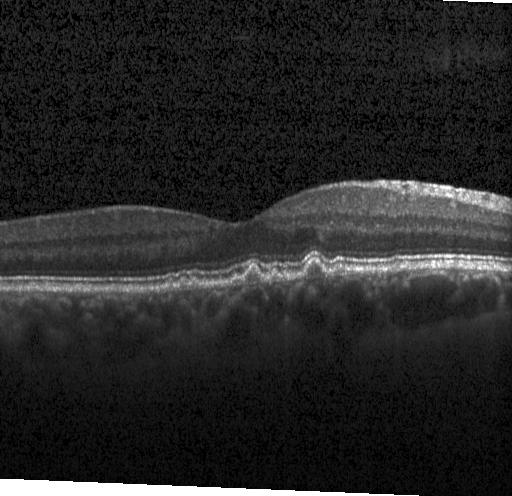

Instrument: Heidelberg Spectralis, fovea-centered, optical coherence tomography B-scan, SD-OCT. Impression: multiple drusen.